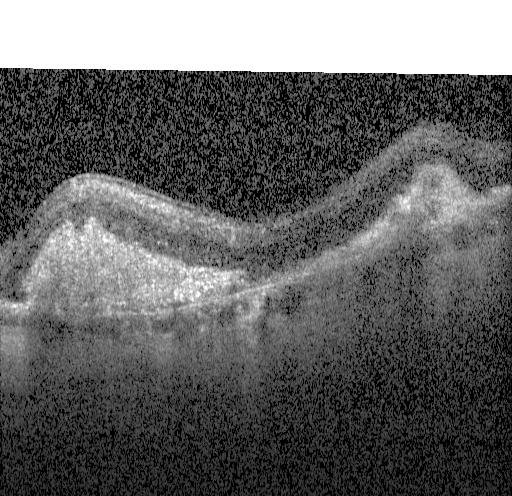
Spectral-domain optical coherence tomography; retinal OCT B-scan; instrument: Heidelberg Spectralis. The scan shows a choroidal neovascular membrane.